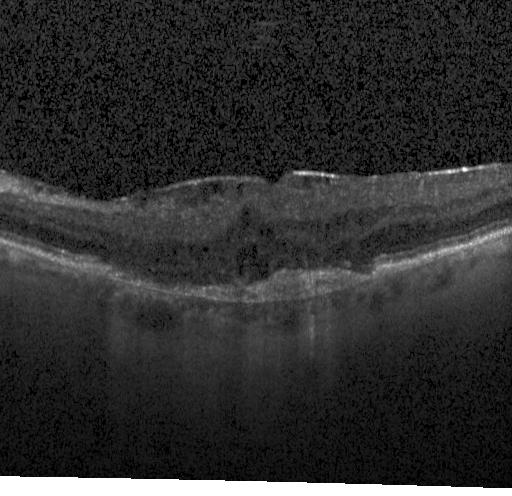
Macular OCT demonstrating a choroidal neovascular membrane.